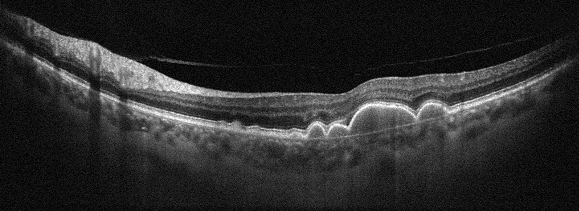
Macular OCT: AMD.